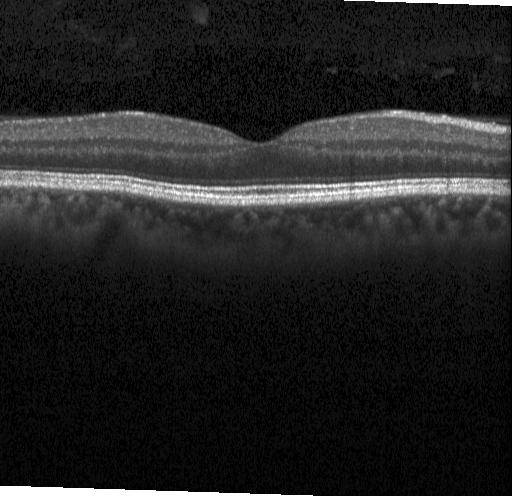 This B-scan demonstrates neither choroidal neovascularization, diabetic macular edema, nor drusen.